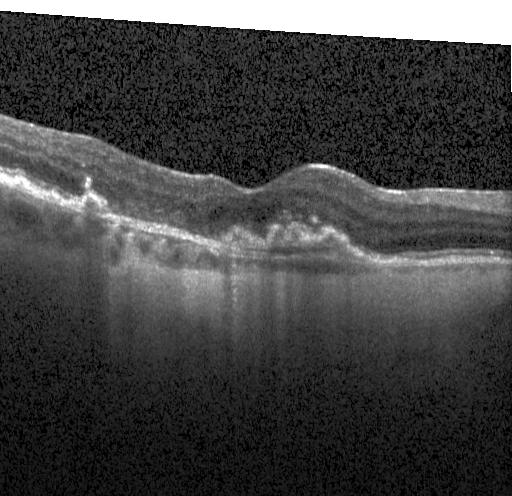

Heidelberg Spectralis · macular scan · SD-OCT · optical coherence tomography B-scan
Choroidal neovascularization.